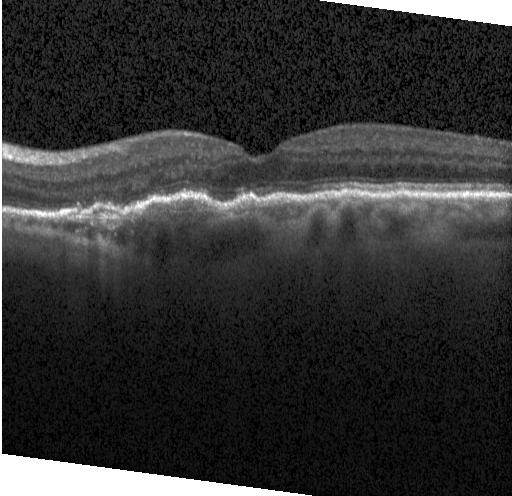
OCT B-scan showing a choroidal neovascular membrane.